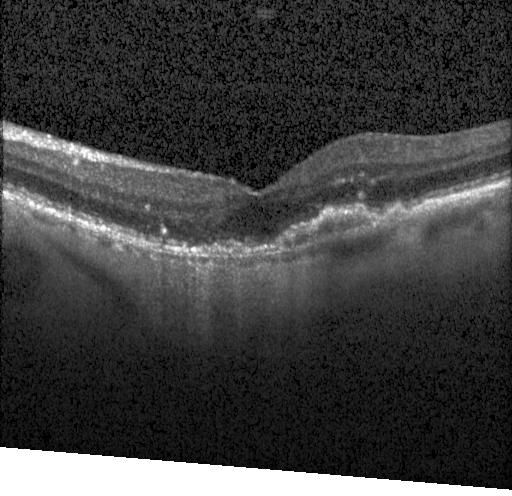 Retinal OCT cross-section showing choroidal neovascularization.